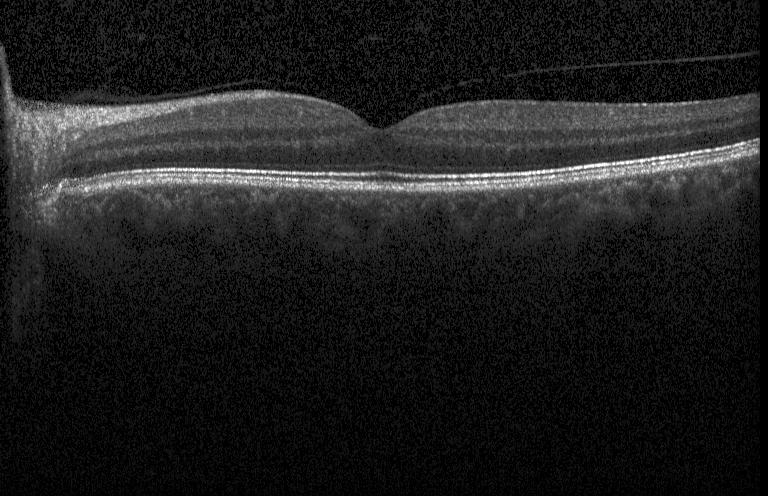 Optical coherence tomography B-scan. Through the macula. Heidelberg Spectralis OCT system. Spectral-domain OCT
Macular OCT: neither choroidal neovascularization, diabetic macular edema, nor drusen.